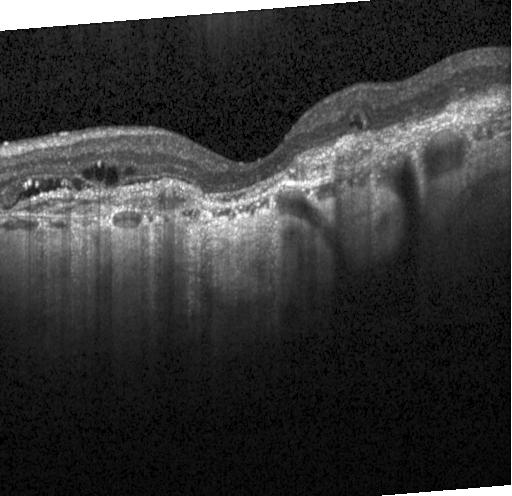
Impression: a choroidal neovascular membrane.